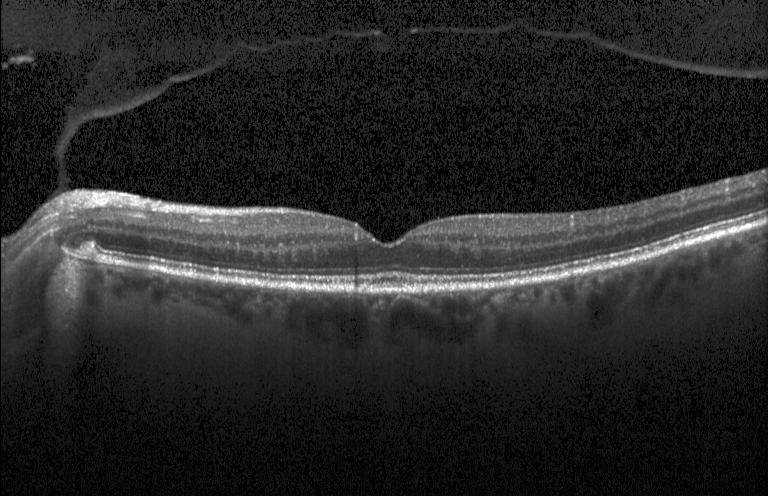

Spectral-domain OCT; instrument: Heidelberg Spectralis; OCT line scan. Dx: no choroidal neovascularization, no diabetic macular edema, and no drusen.